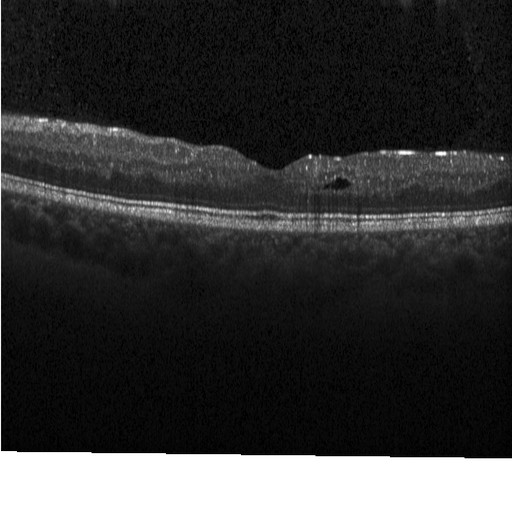
OCT finding: DME.